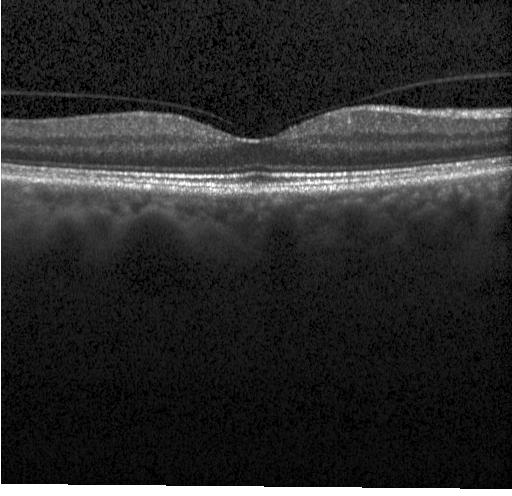
Horizontal scan through the fovea; acquired on a Heidelberg Spectralis; spectral-domain OCT; OCT B-scan.
Finding: no choroidal neovascularization, diabetic macular edema, or drusen.